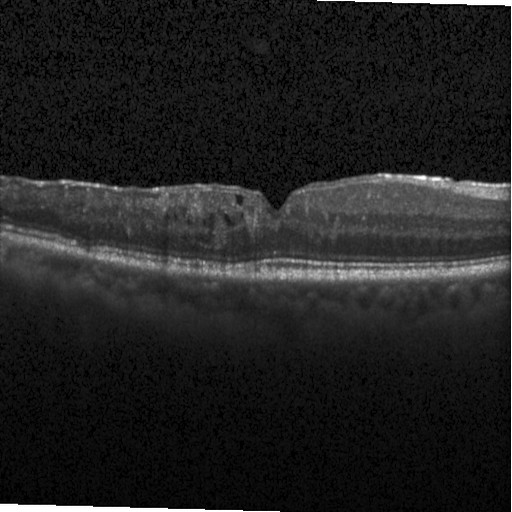
Centered on the fovea. Retinal OCT cross-section. Acquired on a Heidelberg Spectralis.
Diabetic macular edema.